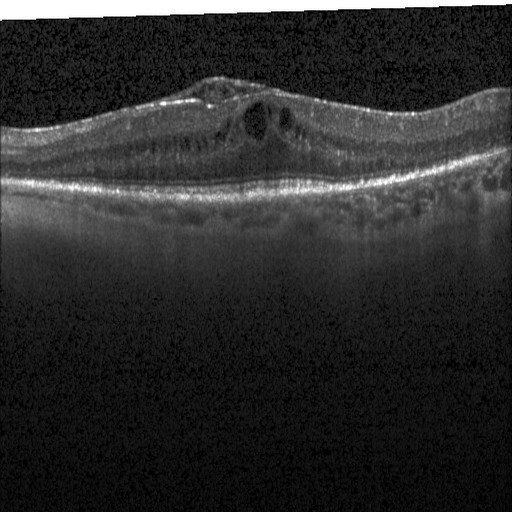 Heidelberg Spectralis OCT system. Optical coherence tomography B-scan. Spectral-domain OCT. Centered on the fovea. Assessment: diabetic macular edema (DME).